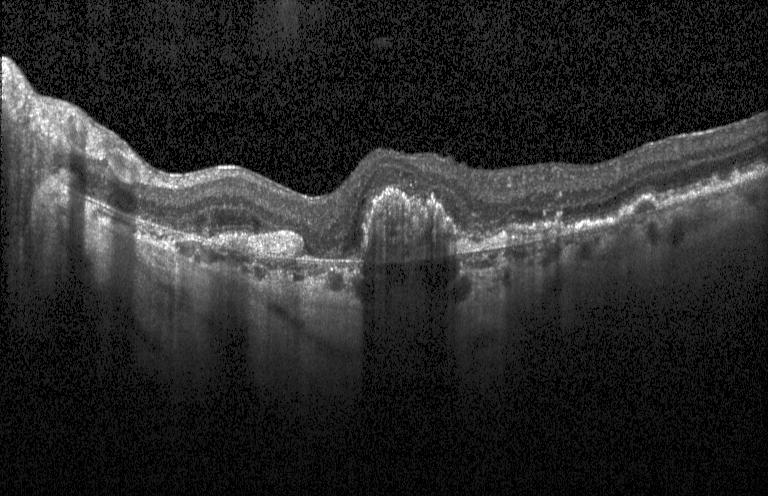
Finding: a choroidal neovascular membrane.